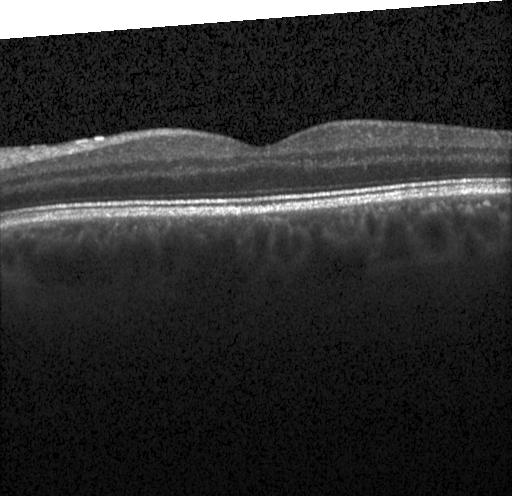 Retinal OCT B-scan
Diagnosis: no evidence of CNV, DME, or drusen.